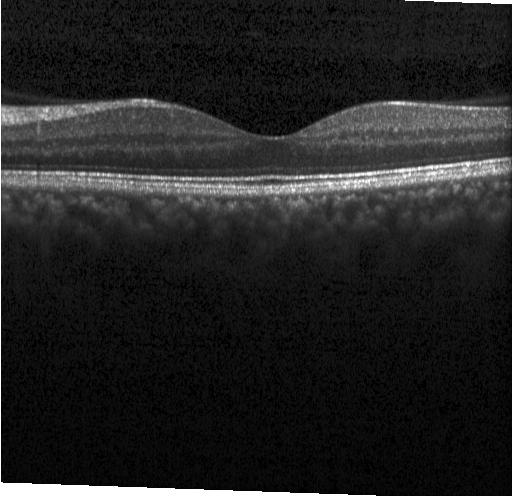
Macular OCT demonstrating no evidence of choroidal neovascularization, diabetic macular edema, or drusen.